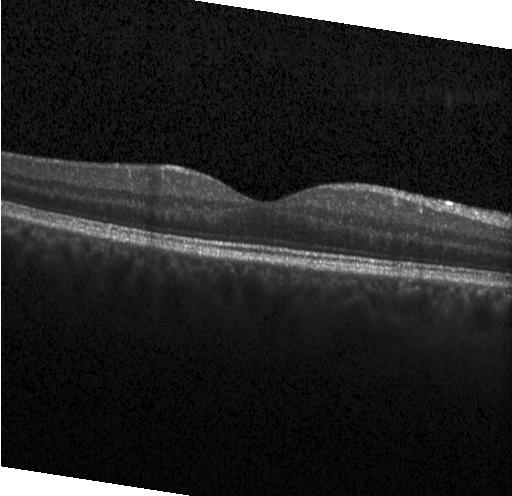
Spectral-domain OCT B-scan: no CNV, no DME, and no drusen.